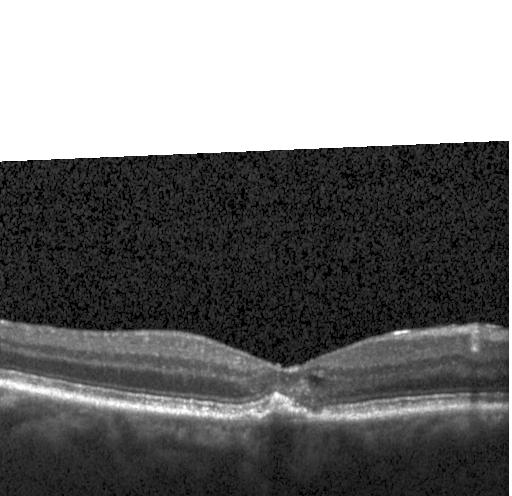
SD-OCT; OCT B-scan; acquired on a Heidelberg Spectralis — Macular OCT: a choroidal neovascular membrane.